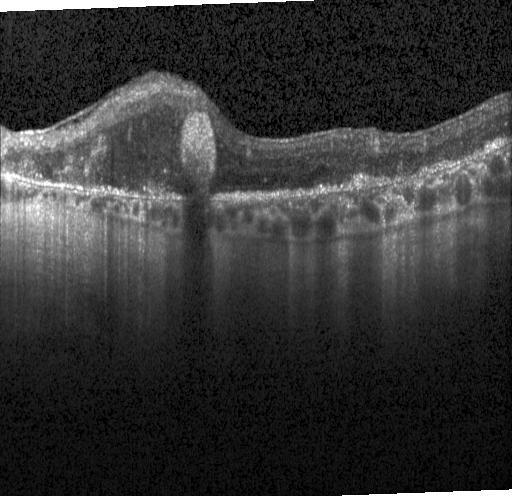 This B-scan demonstrates CNV.